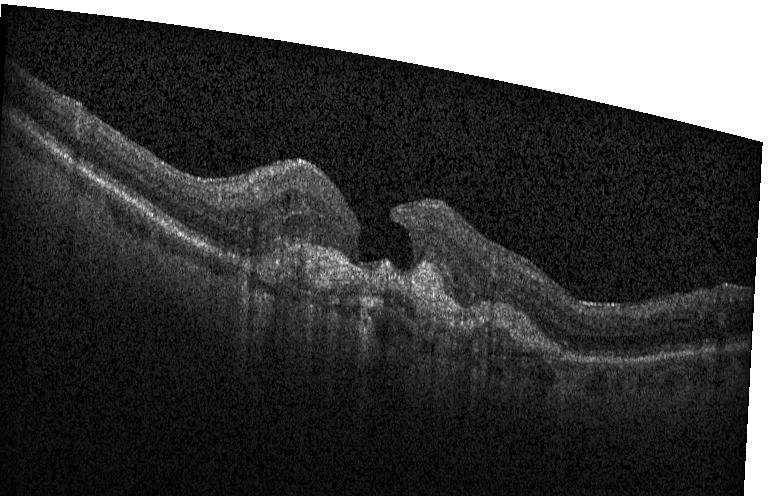
Impression: a choroidal neovascular membrane.